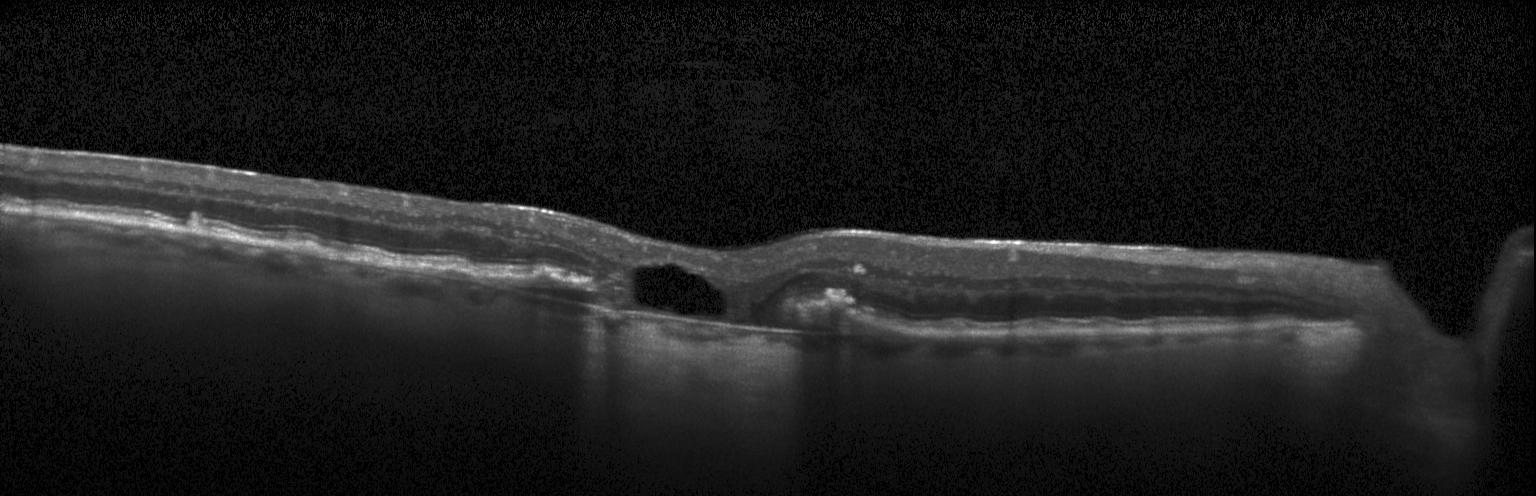 Heidelberg Spectralis OCT system. Retinal OCT B-scan. Fovea-centered
This B-scan demonstrates choroidal neovascularization (CNV).